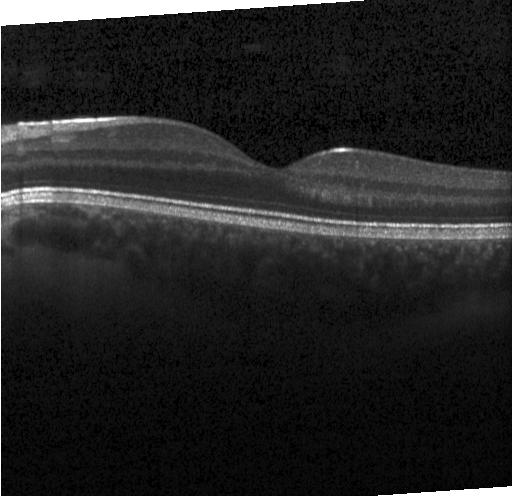
Finding: no choroidal neovascularization, diabetic macular edema, or drusen.